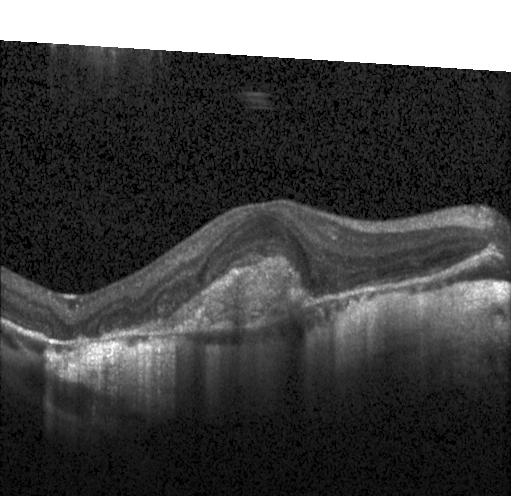
OCT line scan.
Choroidal neovascularization (CNV).